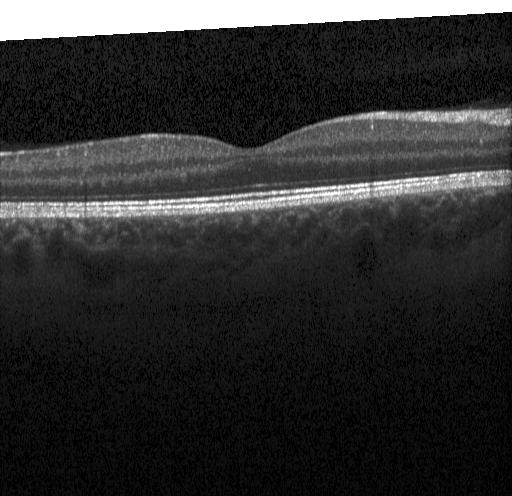 Diagnosis: neither CNV, DME, nor drusen.